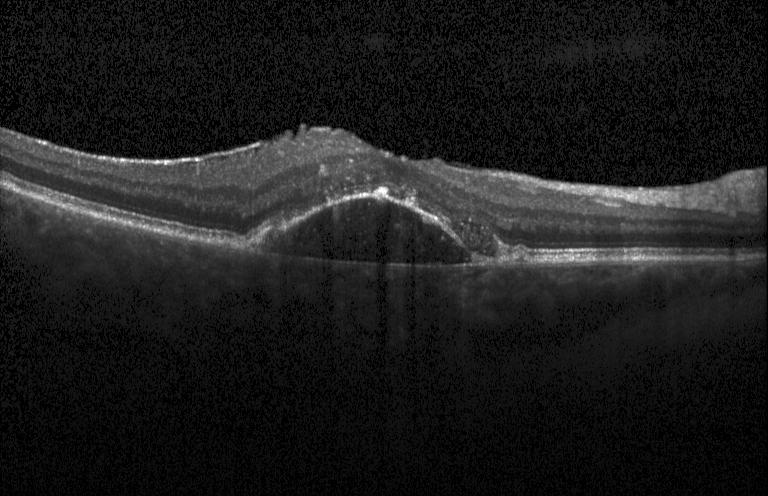 Impression: a choroidal neovascular membrane.